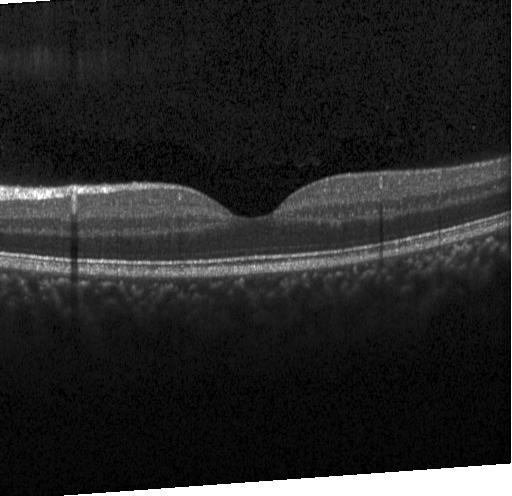 Macular OCT: no choroidal neovascularization, no diabetic macular edema, and no drusen.